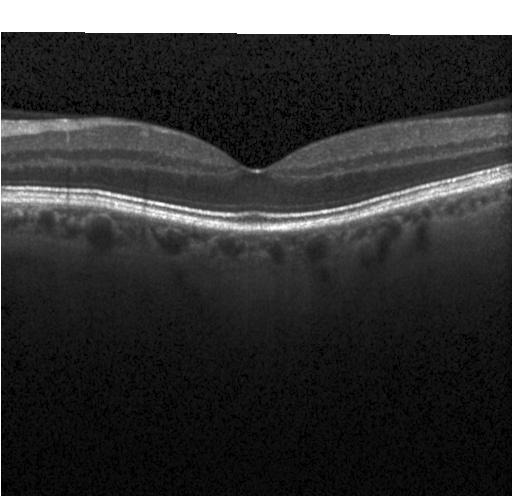
Retinal OCT B-scan. Heidelberg Spectralis
Macular OCT: no choroidal neovascularization, no diabetic macular edema, and no drusen.